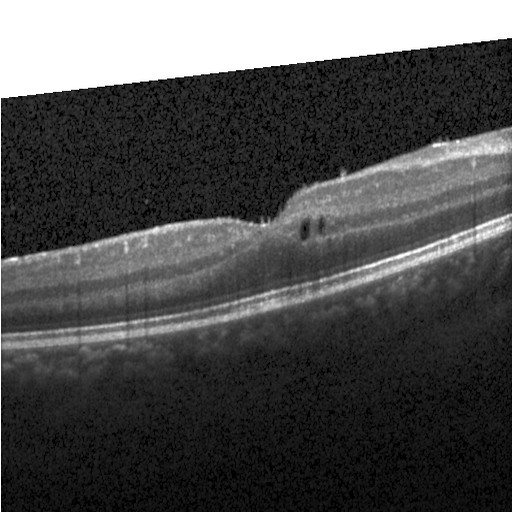

Optical coherence tomography B-scan. Instrument: Heidelberg Spectralis. This B-scan demonstrates diabetic macular edema (DME).